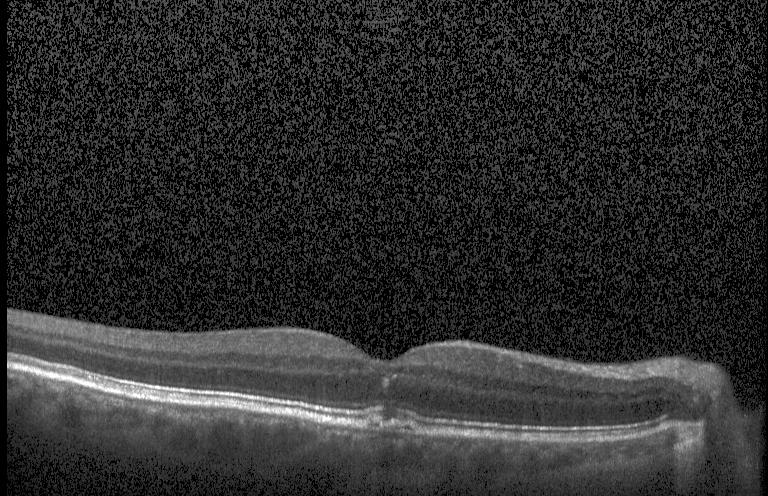
Optical coherence tomography B-scan, spectral-domain OCT, horizontal scan through the fovea — Finding: choroidal neovascularization.